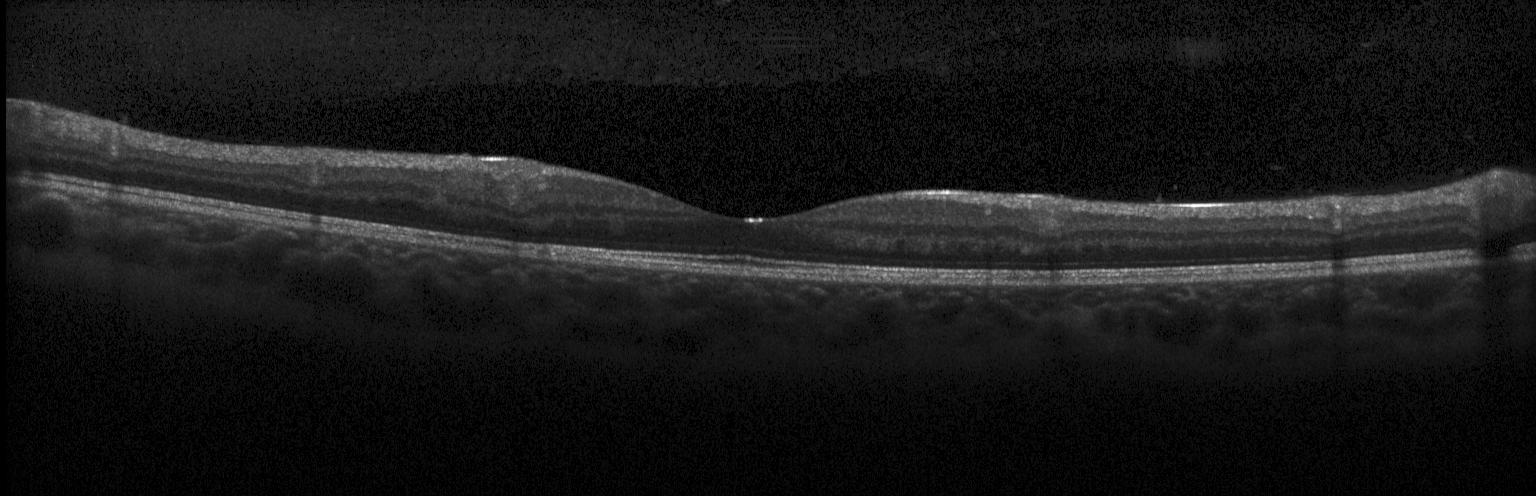
Neither choroidal neovascularization, diabetic macular edema, nor drusen.